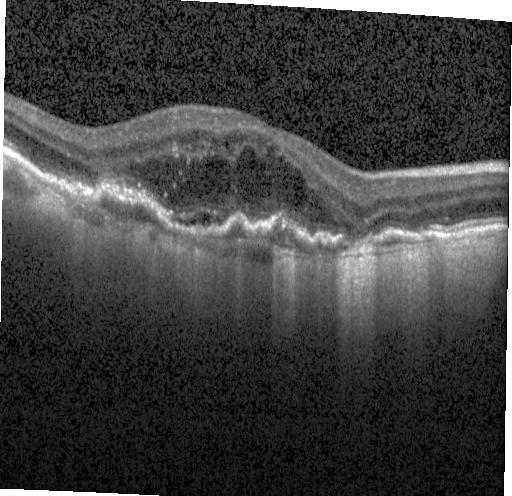 SD-OCT, OCT line scan, through the macula, acquired on a Heidelberg Spectralis. Finding: a choroidal neovascular membrane.